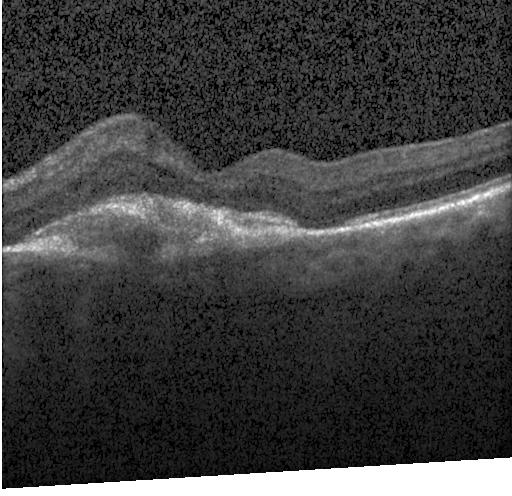
Instrument: Heidelberg Spectralis. Optical coherence tomography B-scan. Spectral-domain OCT. Fovea-centered
Finding: choroidal neovascularization.